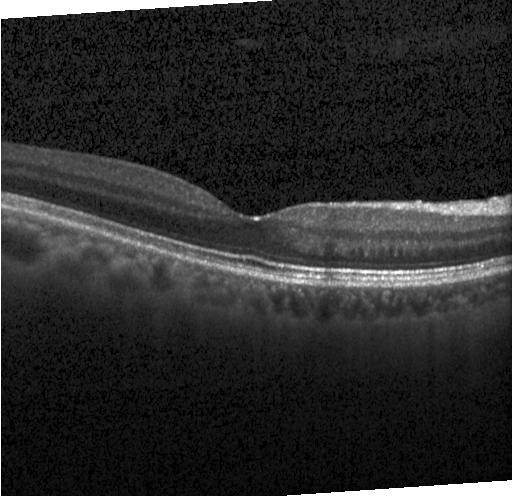

OCT B-scan. Finding: no choroidal neovascularization, diabetic macular edema, or drusen.